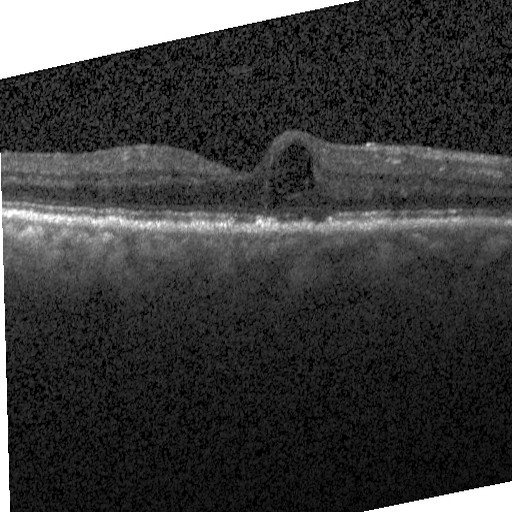
Optical coherence tomography B-scan — This B-scan demonstrates diabetic macular edema (DME).